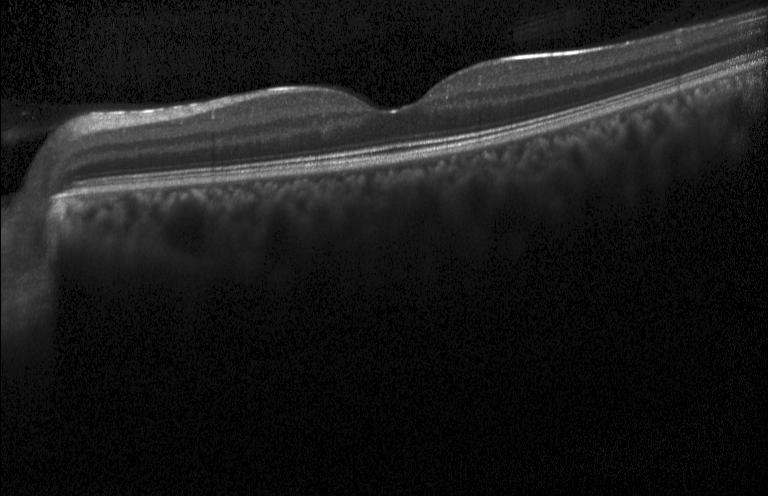 Diagnosis: no choroidal neovascularization, no diabetic macular edema, and no drusen.